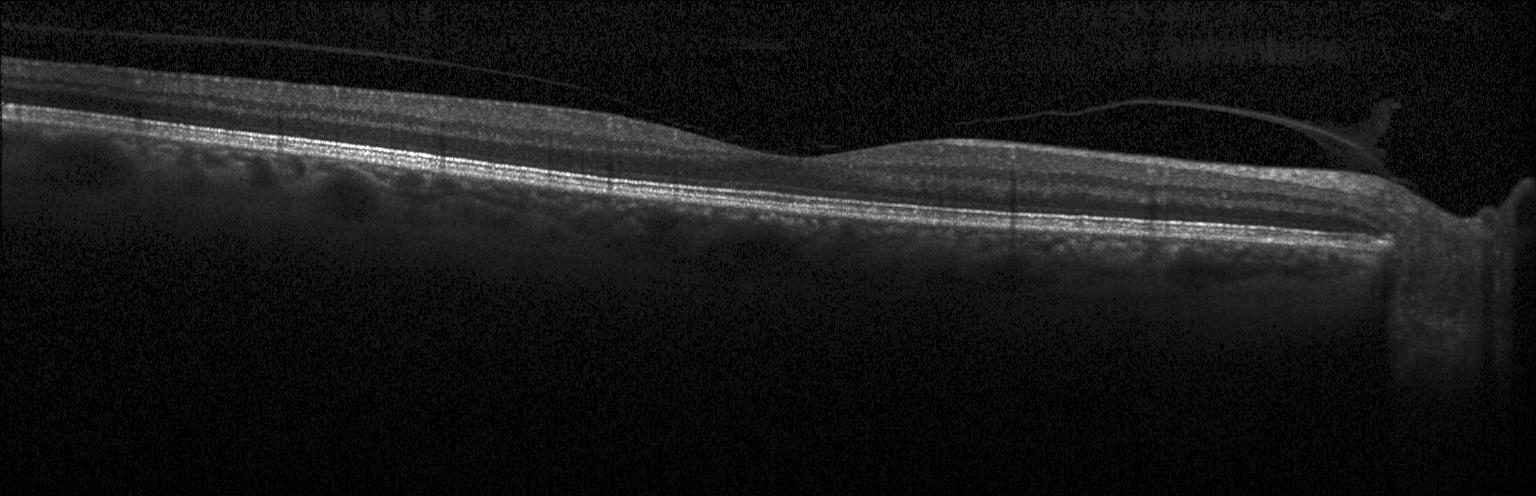 OCT B-scan
Diagnosis: no evidence of choroidal neovascularization, diabetic macular edema, or drusen.